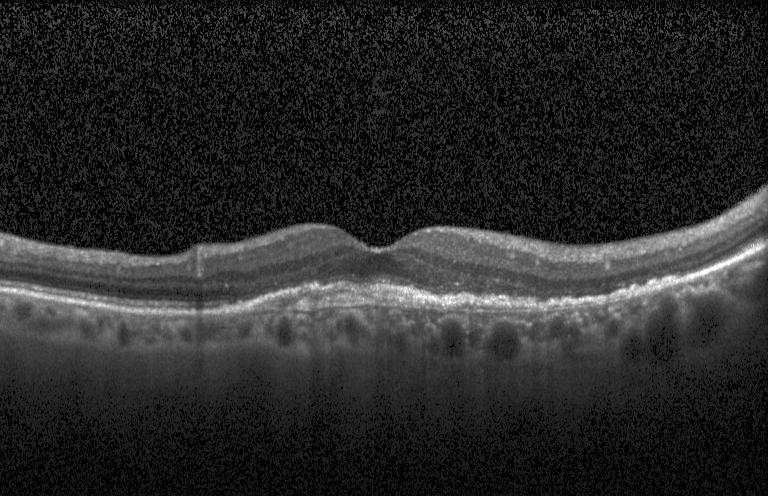
Impression: a choroidal neovascular membrane.